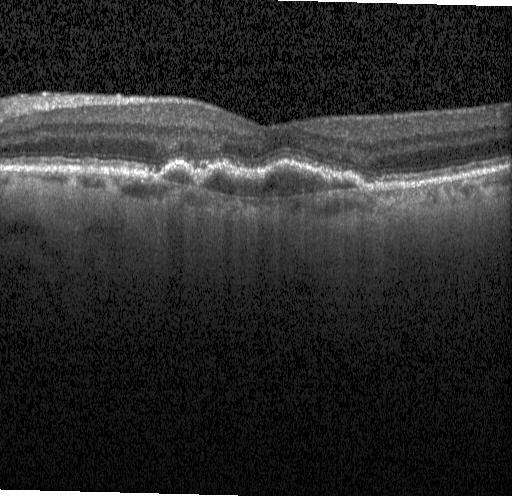
OCT line scan; centered on the fovea; spectral-domain optical coherence tomography; instrument: Heidelberg Spectralis.
Finding: CNV.